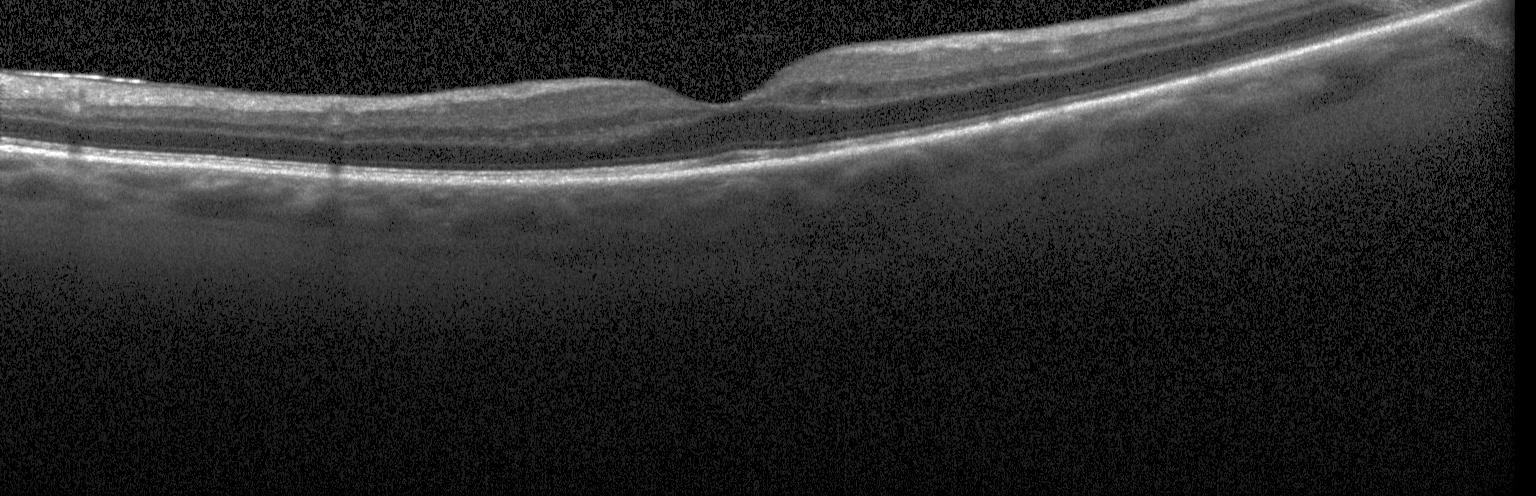 Acquired on a Heidelberg Spectralis · OCT line scan — This B-scan demonstrates no choroidal neovascularization, diabetic macular edema, or drusen.